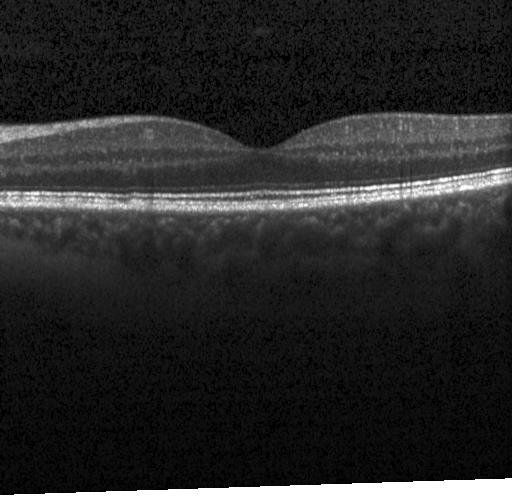

Macular OCT demonstrating neither choroidal neovascularization, diabetic macular edema, nor drusen.